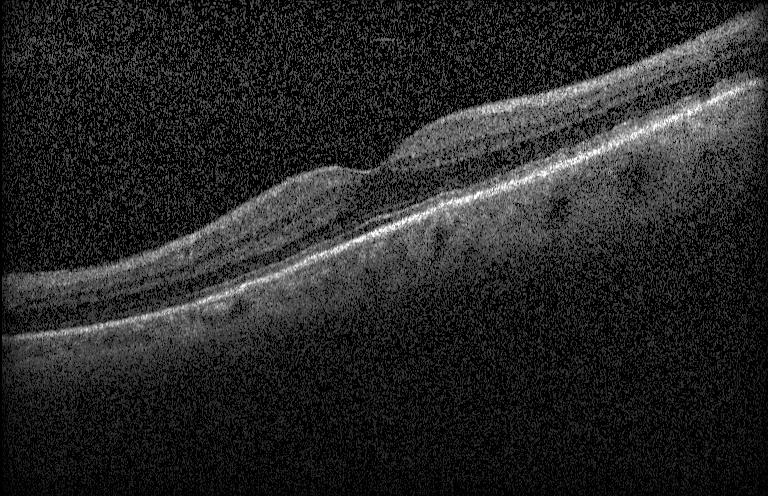

Finding: no choroidal neovascularization, diabetic macular edema, or drusen.